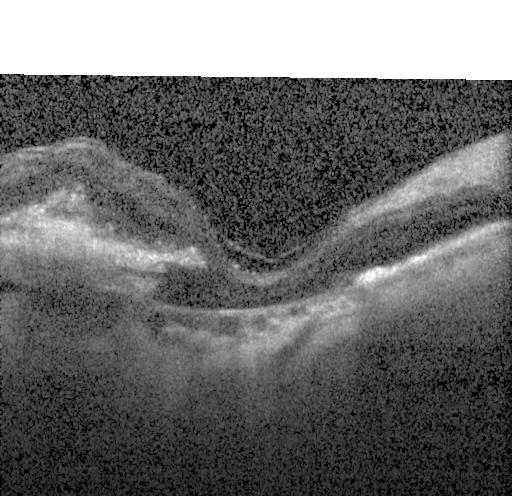

Optical coherence tomography scan. Spectral-domain OCT. Macular scan
Assessment: a choroidal neovascular membrane.